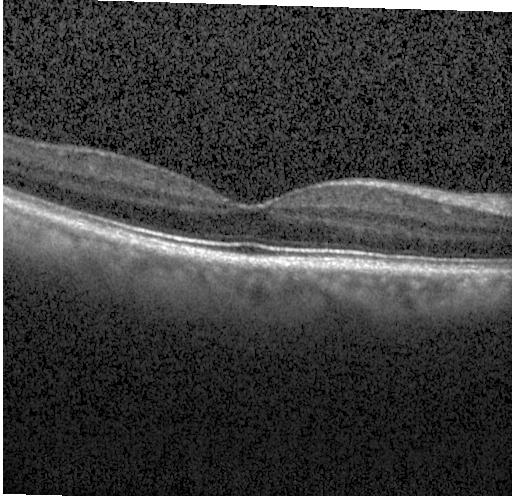

Instrument: Heidelberg Spectralis. Through the macula. Optical coherence tomography B-scan. Spectral-domain optical coherence tomography
Diagnosis: no CNV, DME, or drusen.